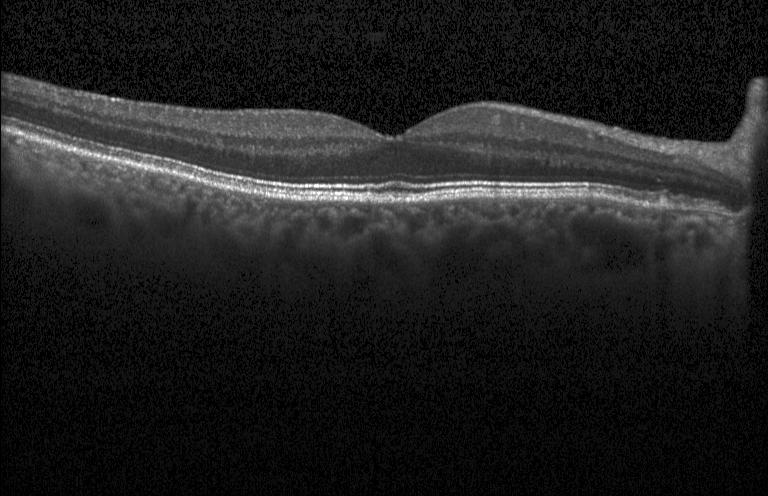 Horizontal scan through the fovea. SD-OCT. Retinal OCT cross-section. Heidelberg Spectralis OCT system. This B-scan demonstrates neither choroidal neovascularization, diabetic macular edema, nor drusen.